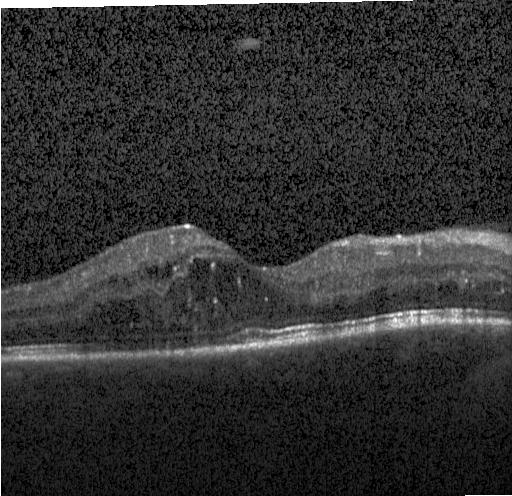

Impression: diabetic macular edema (DME).